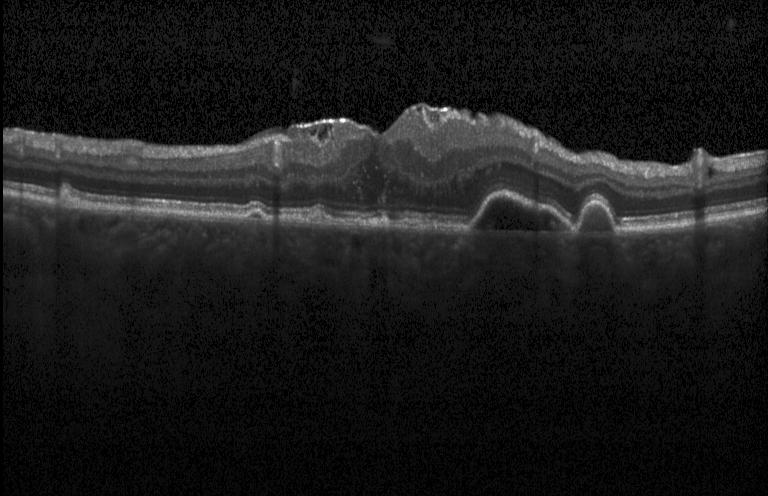 Retinal OCT B-scan. Instrument: Heidelberg Spectralis. Through the macula
Finding: choroidal neovascularization.